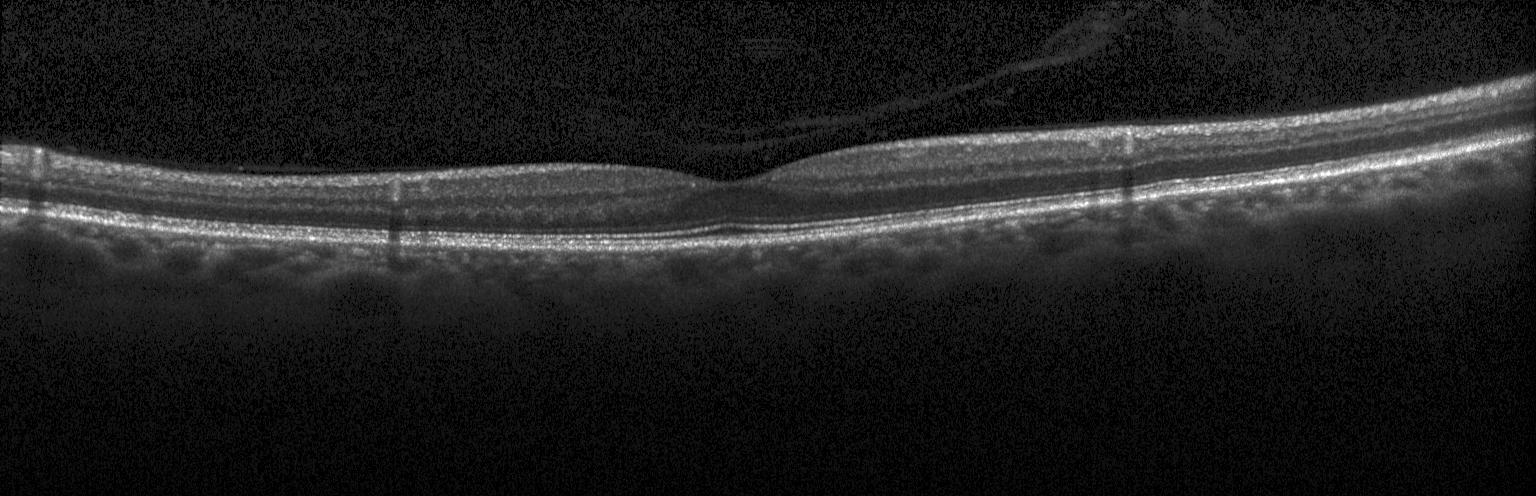

Finding: no evidence of choroidal neovascularization, diabetic macular edema, or drusen.